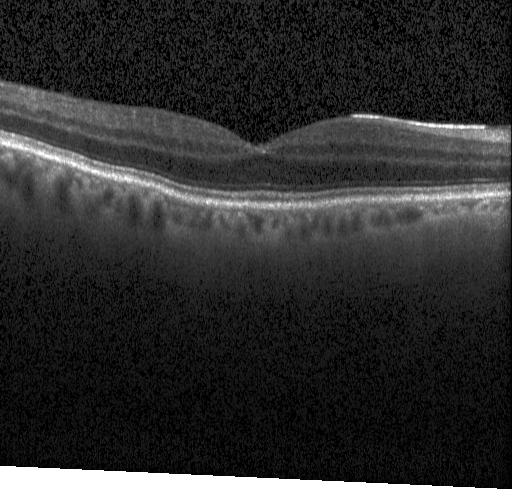 Optical coherence tomography B-scan; through the macula; spectral-domain optical coherence tomography; instrument: Heidelberg Spectralis.
Impression: neither choroidal neovascularization, diabetic macular edema, nor drusen.